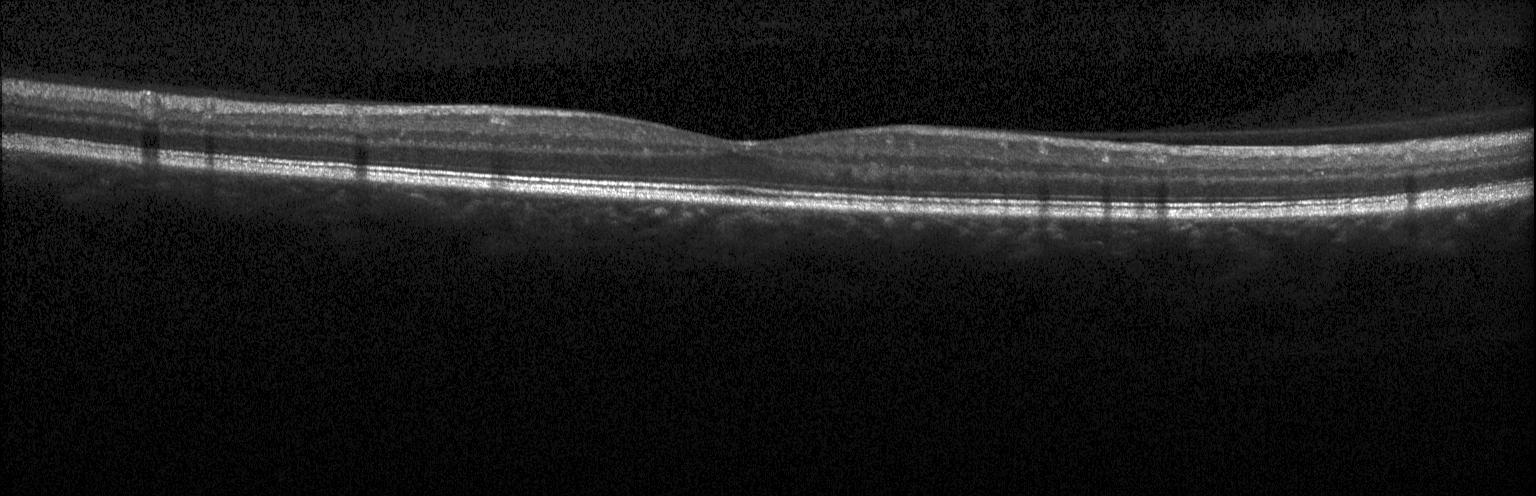

Horizontal scan through the fovea; SD-OCT; instrument: Heidelberg Spectralis; OCT B-scan
Diagnosis: no evidence of choroidal neovascularization, diabetic macular edema, or drusen.